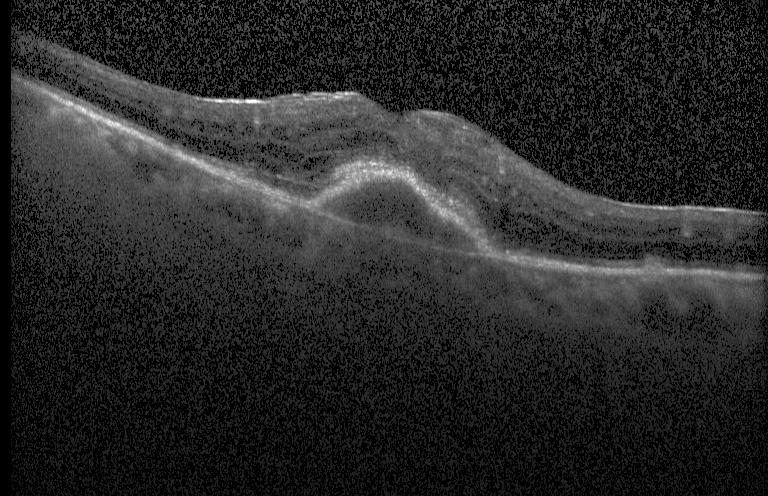

Heidelberg Spectralis OCT system. OCT line scan.
Finding: choroidal neovascularization (CNV).